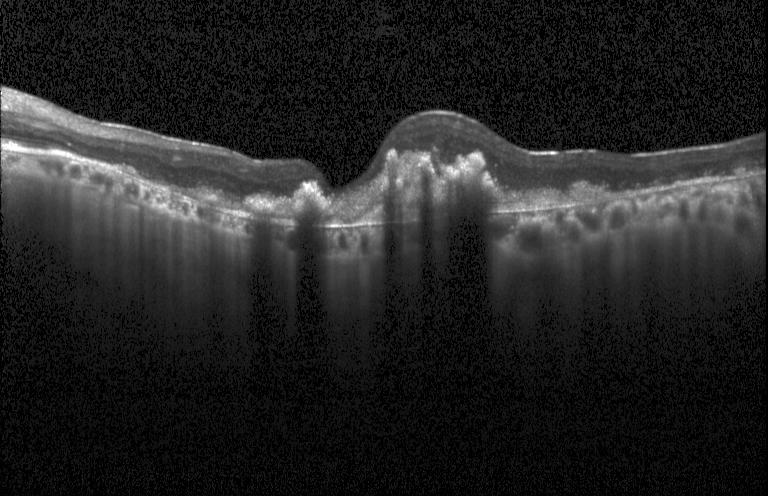

OCT B-scan showing choroidal neovascularization (CNV).